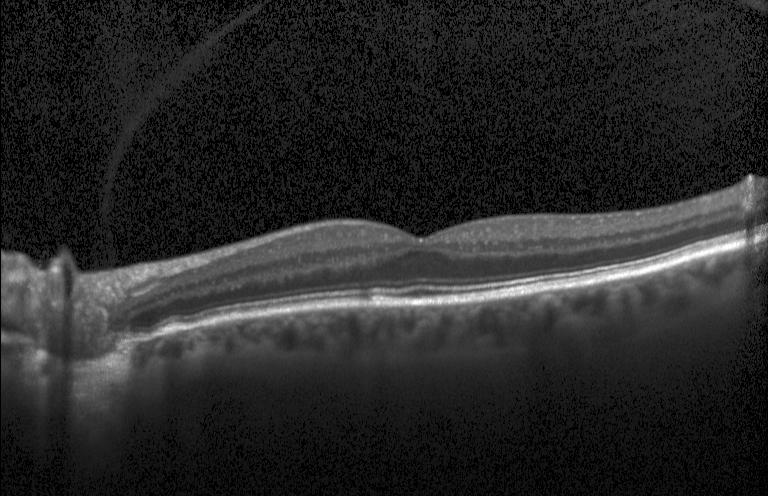 This B-scan demonstrates no choroidal neovascularization, no diabetic macular edema, and no drusen.